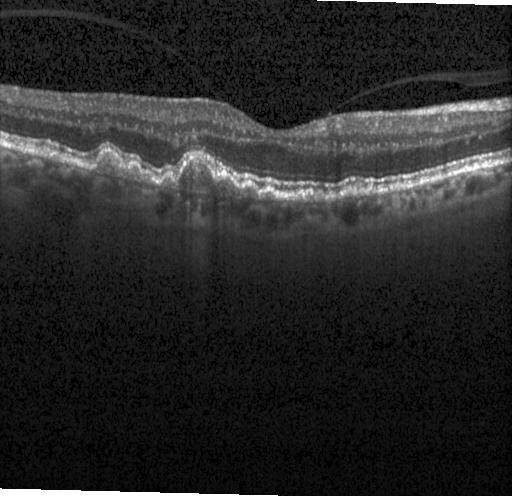
Optical coherence tomography B-scan. Diagnosis: multiple drusen.